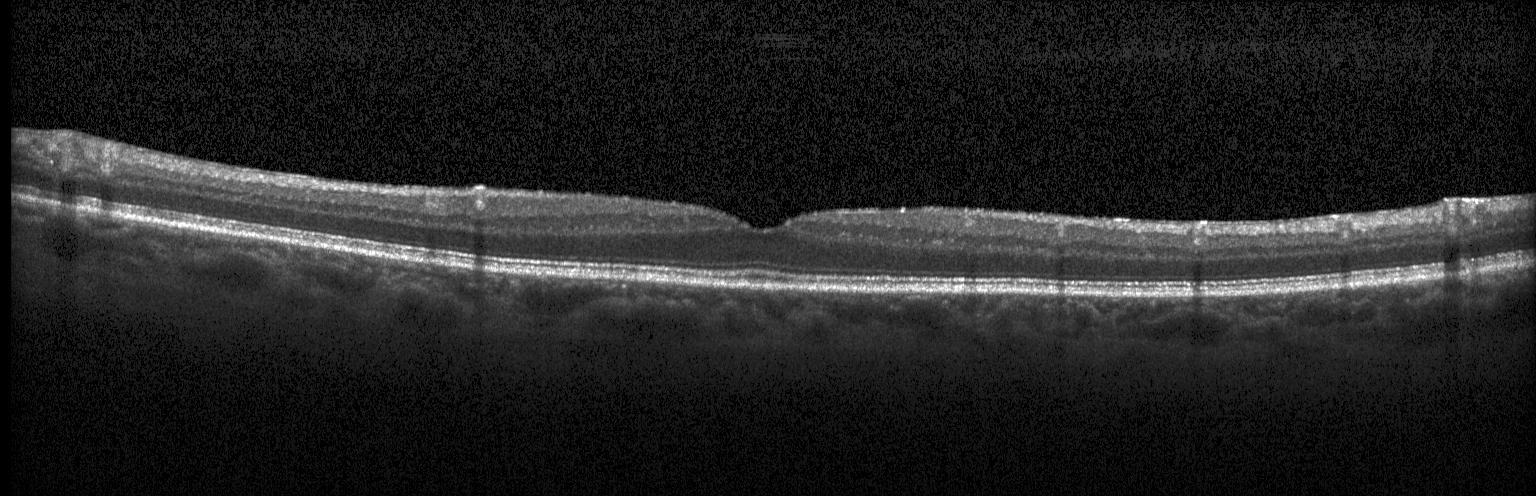 OCT B-scan. Impression: no CNV, no DME, and no drusen.